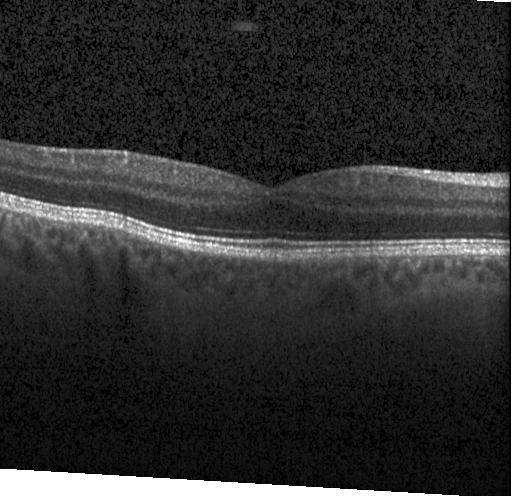
Heidelberg Spectralis · optical coherence tomography B-scan. This B-scan demonstrates no CNV, no DME, and no drusen.